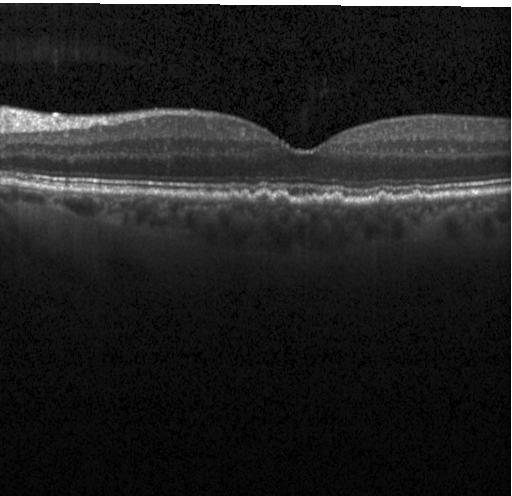
Heidelberg Spectralis. Optical coherence tomography B-scan
OCT finding: sub-RPE drusenoid deposits.